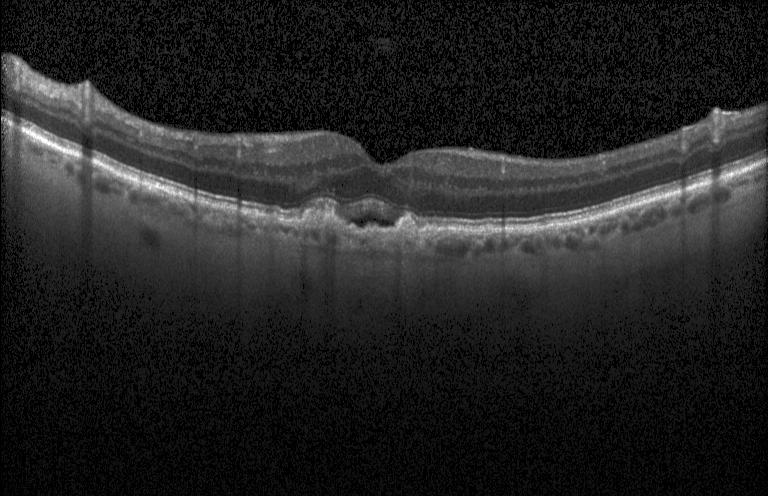 Retinal OCT B-scan. Choroidal neovascularization.